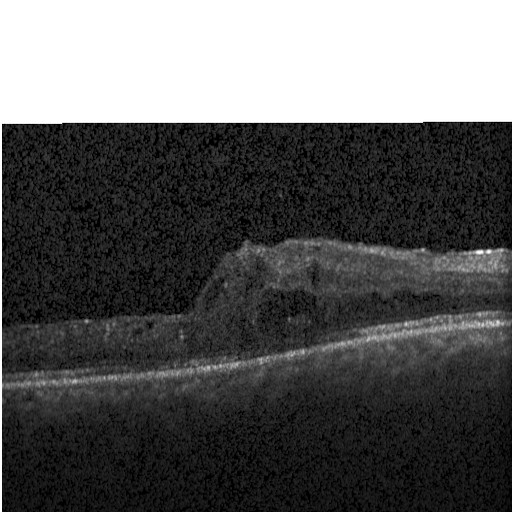
Retinal OCT cross-section, centered on the fovea — Impression: diabetic macular edema.